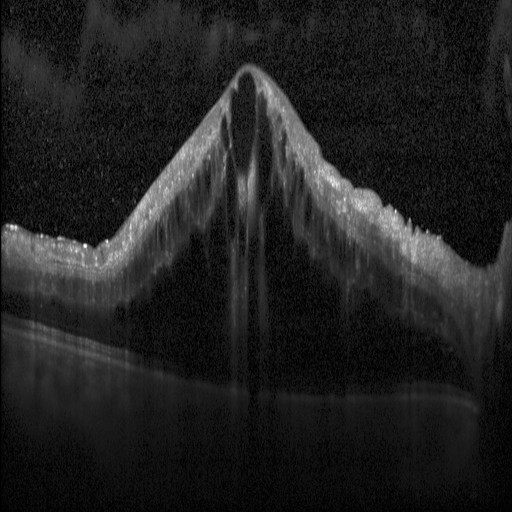
Assessment: diabetic macular edema (DME).